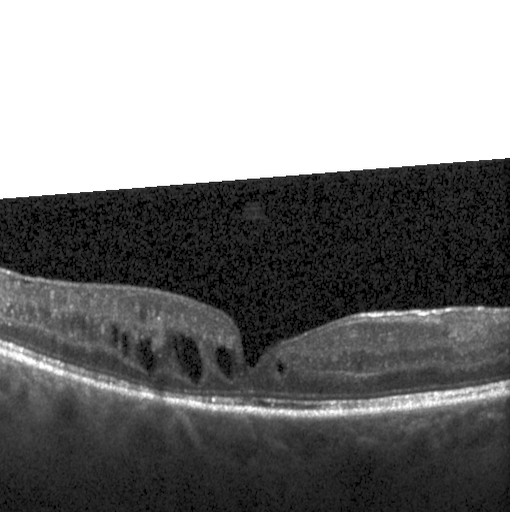

This B-scan demonstrates diabetic macular edema.